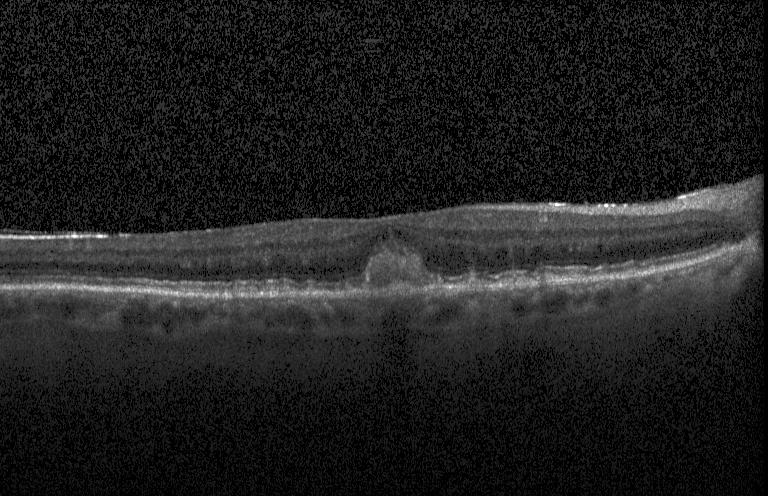
Fovea-centered · optical coherence tomography B-scan — Finding: a choroidal neovascular membrane.